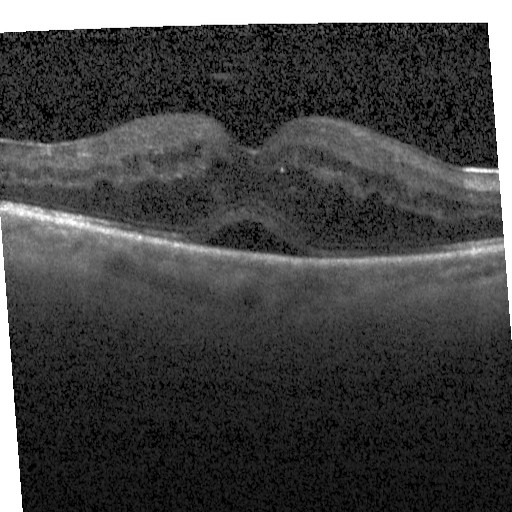 Macular OCT demonstrating DME.